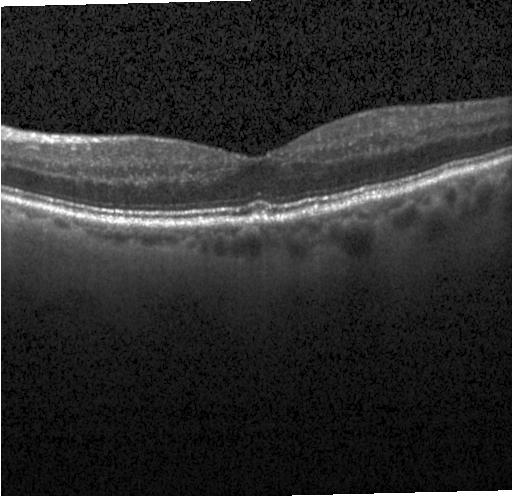

Centered on the fovea. Retinal OCT cross-section. Spectral-domain OCT
Impression: multiple drusen.